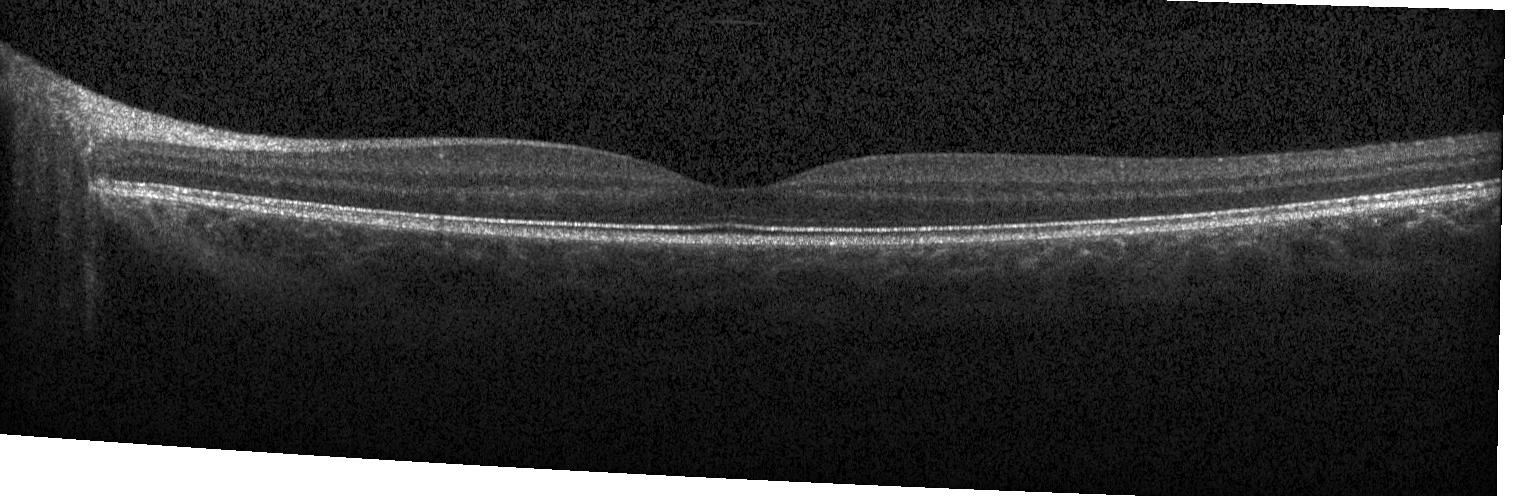
Instrument: Heidelberg Spectralis. Spectral-domain optical coherence tomography. Fovea-centered. Optical coherence tomography scan — This B-scan demonstrates no evidence of choroidal neovascularization, diabetic macular edema, or drusen.